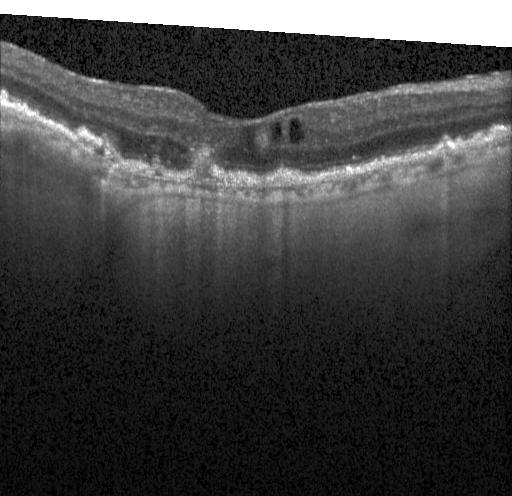
OCT line scan. OCT finding: choroidal neovascularization (CNV).